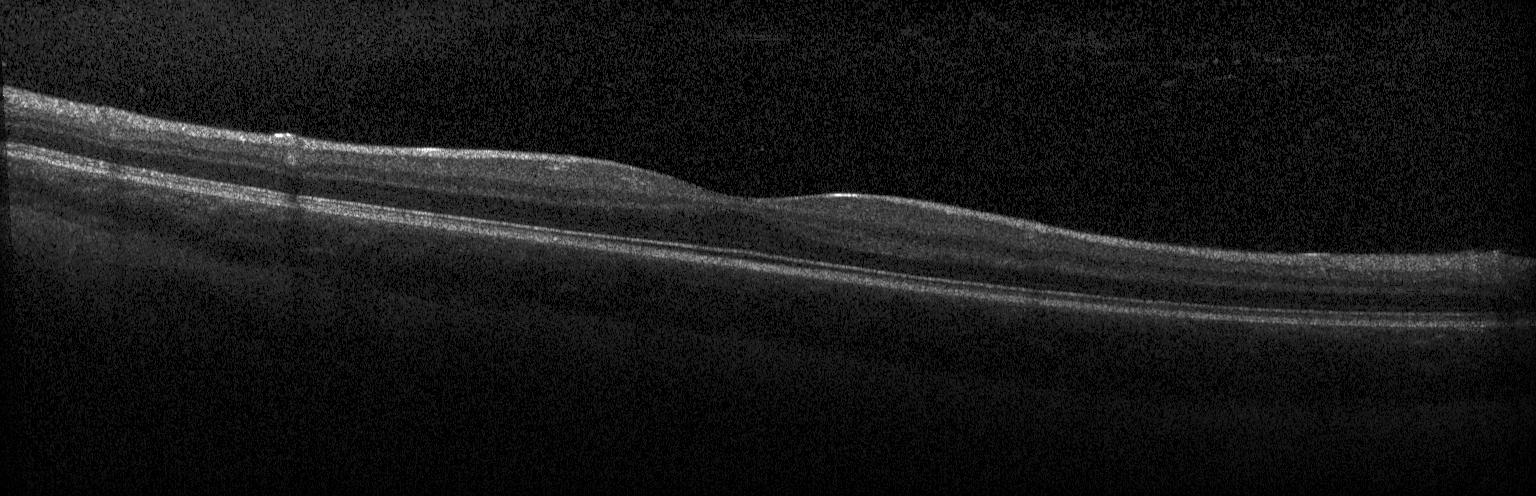
Dx: neither CNV, DME, nor drusen.